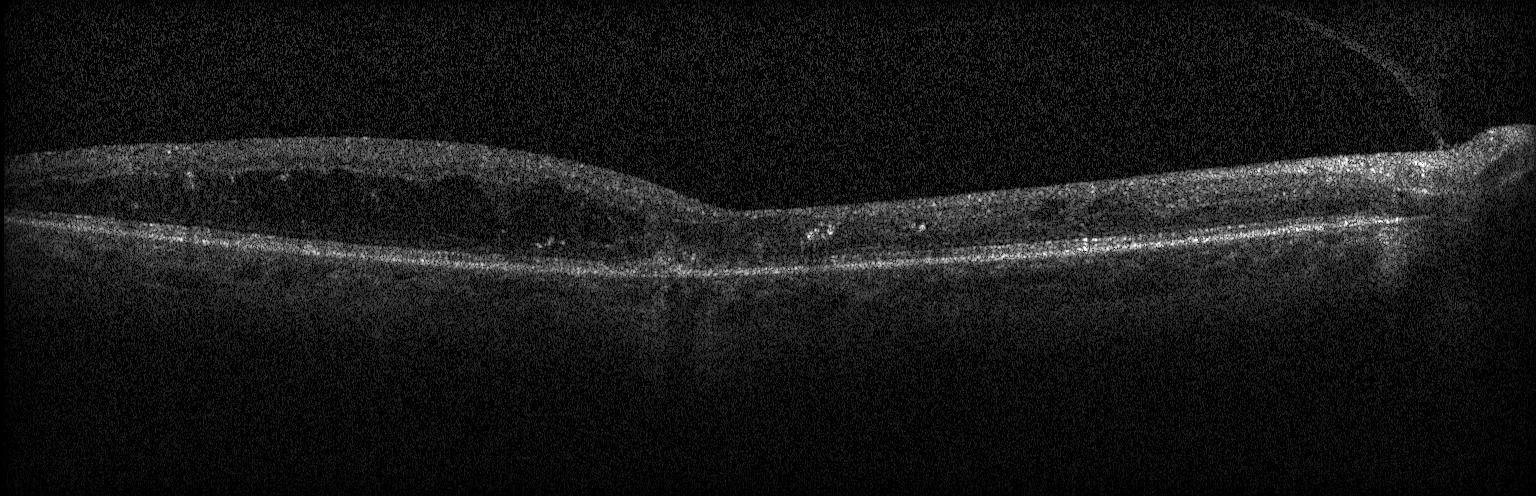

Fovea-centered · OCT B-scan
Finding: DME.